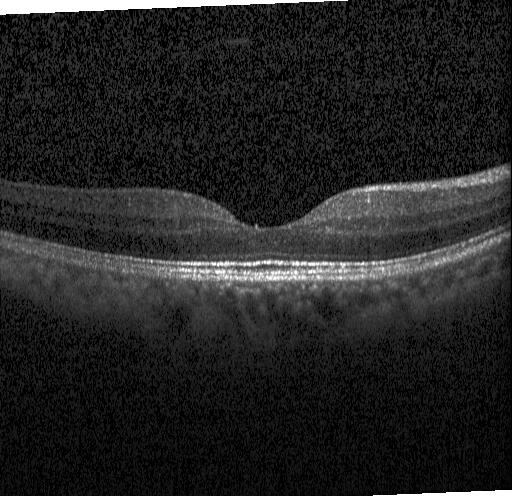
OCT line scan.
Impression: no choroidal neovascularization, no diabetic macular edema, and no drusen.